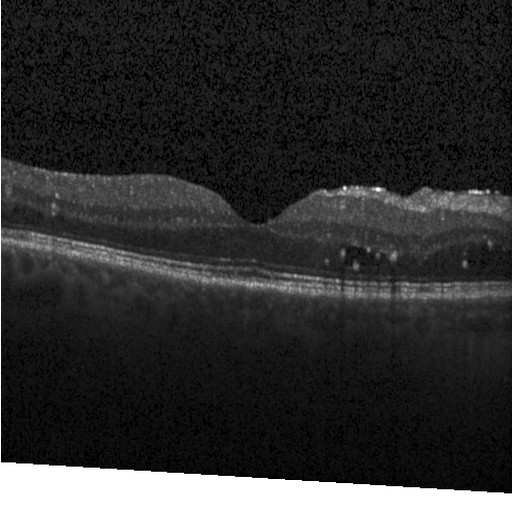 Spectral-domain optical coherence tomography; OCT line scan
Diagnosis: DME.